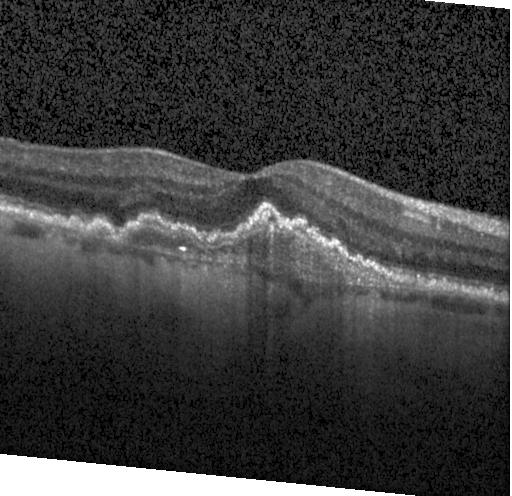
Macular OCT: choroidal neovascularization (CNV).